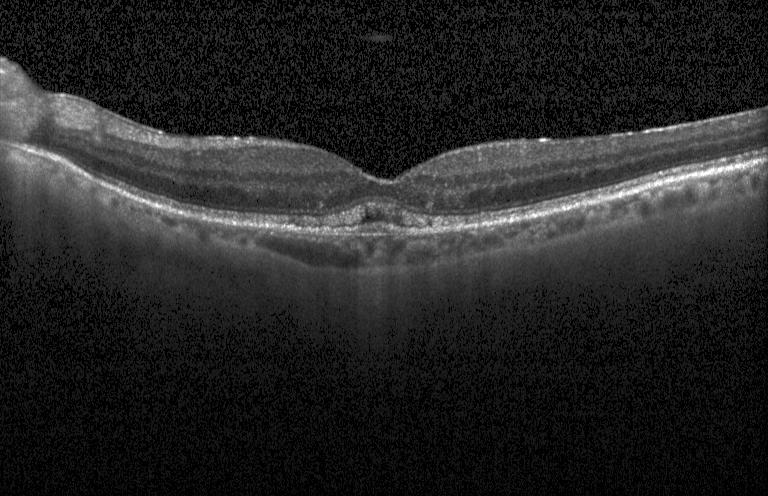 Instrument: Heidelberg Spectralis. Optical coherence tomography B-scan.
Assessment: choroidal neovascularization (CNV).